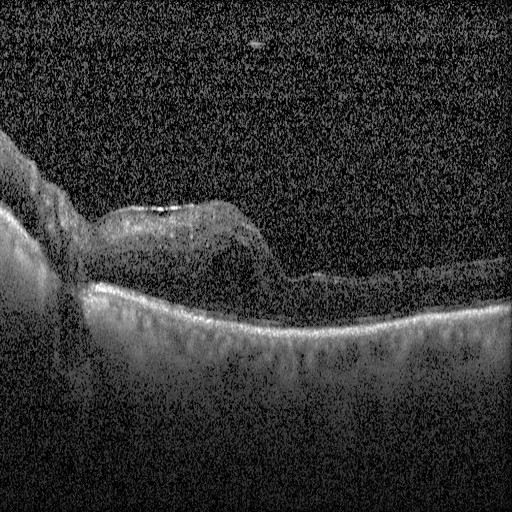
Centered on the fovea; spectral-domain optical coherence tomography; retinal OCT cross-section
Impression: diabetic macular edema (DME).